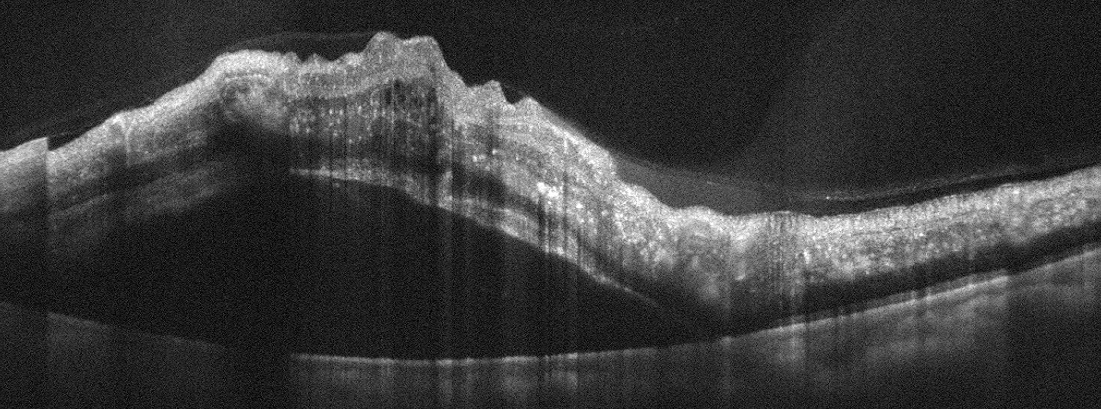 Macular scan · Optovue Avanti RTVue XR · OCT line scan — Finding: retinal vein occlusion.